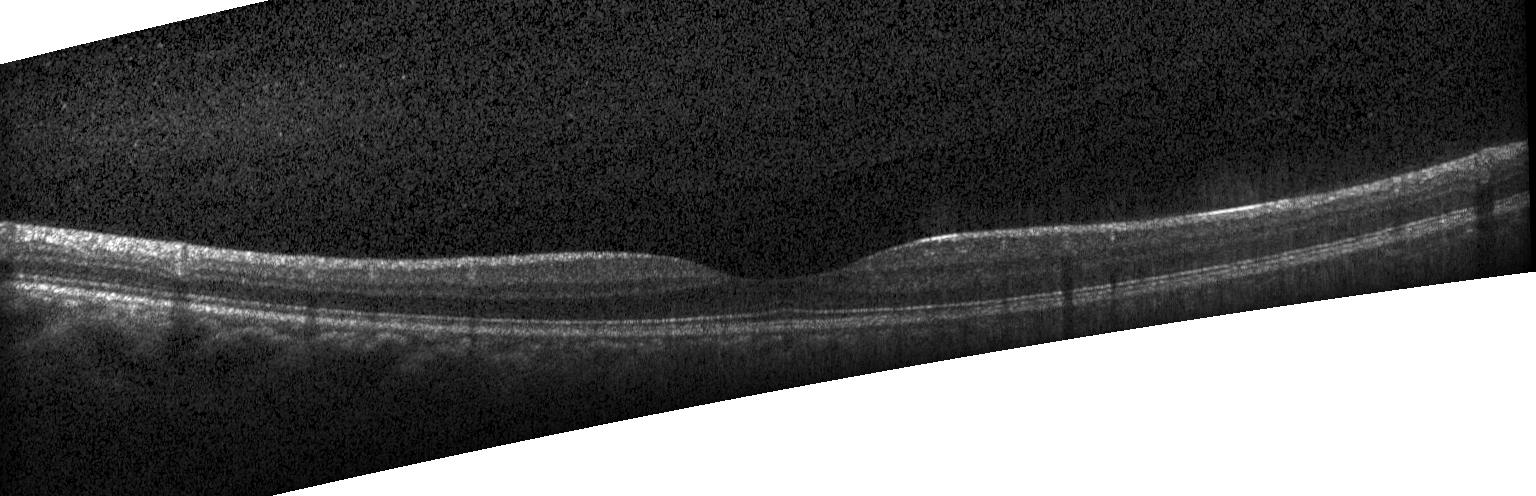
Optical coherence tomography scan. Diagnosis: no evidence of choroidal neovascularization, diabetic macular edema, or drusen.